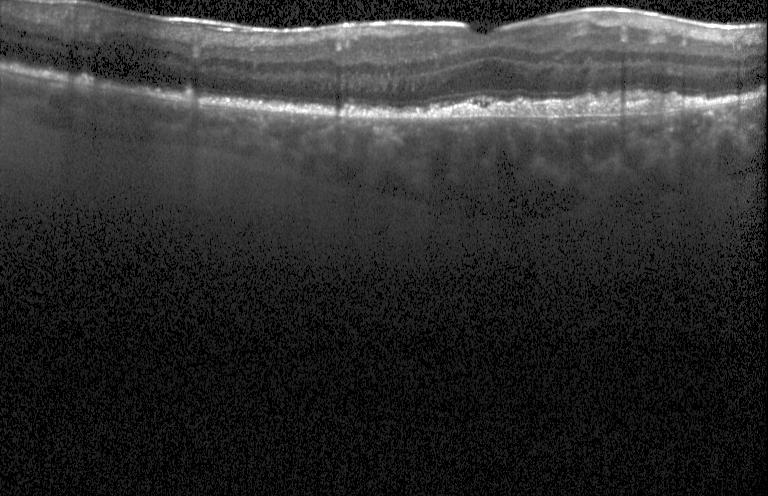
OCT B-scan showing choroidal neovascularization.